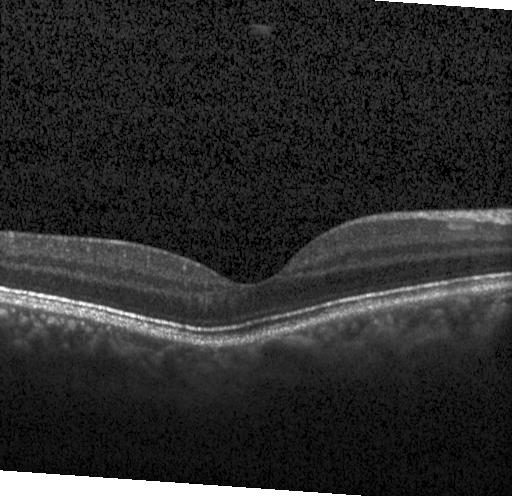 Optical coherence tomography scan; Heidelberg Spectralis OCT system. OCT finding: neither choroidal neovascularization, diabetic macular edema, nor drusen.